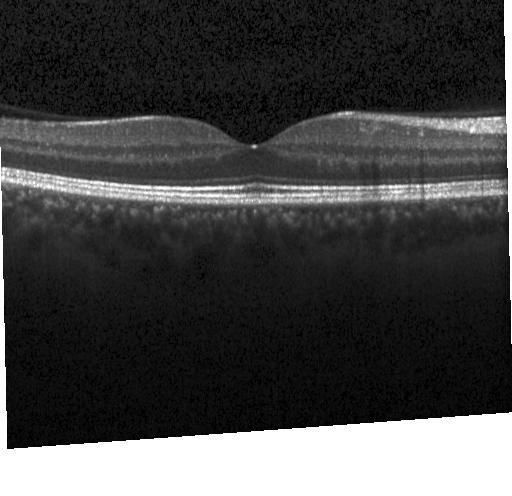 OCT finding: no choroidal neovascularization, no diabetic macular edema, and no drusen.